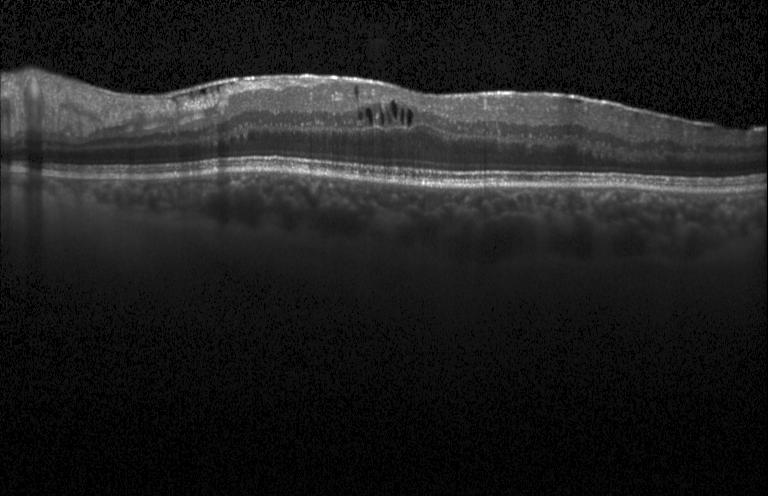
Heidelberg Spectralis · spectral-domain optical coherence tomography · fovea-centered · OCT B-scan
OCT finding: diabetic macular edema.